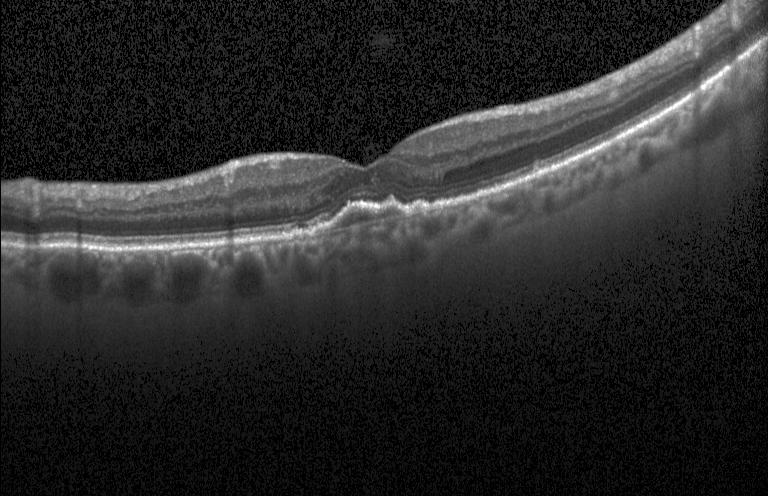

Fovea-centered, Heidelberg Spectralis, OCT B-scan. Finding: a choroidal neovascular membrane.